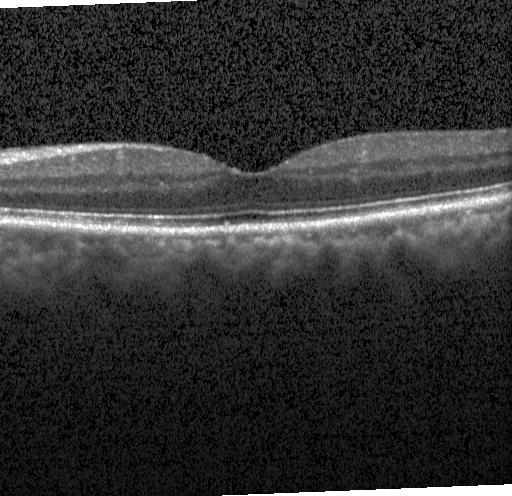

Optical coherence tomography scan — OCT finding: no choroidal neovascularization, no diabetic macular edema, and no drusen.